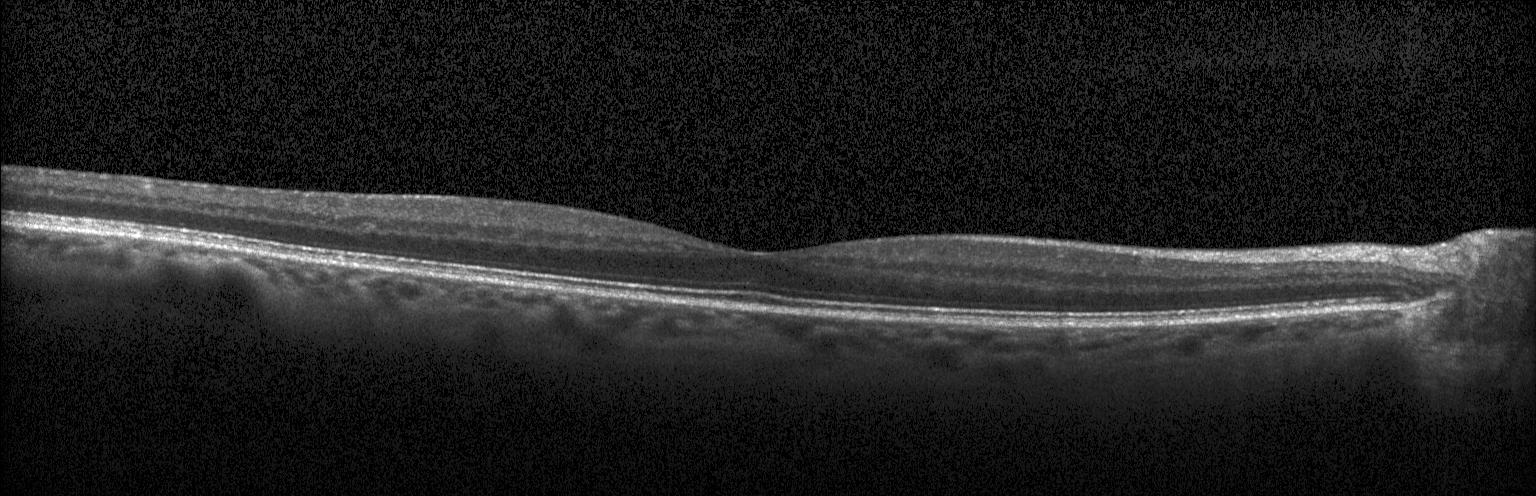

OCT B-scan showing no choroidal neovascularization, no diabetic macular edema, and no drusen.